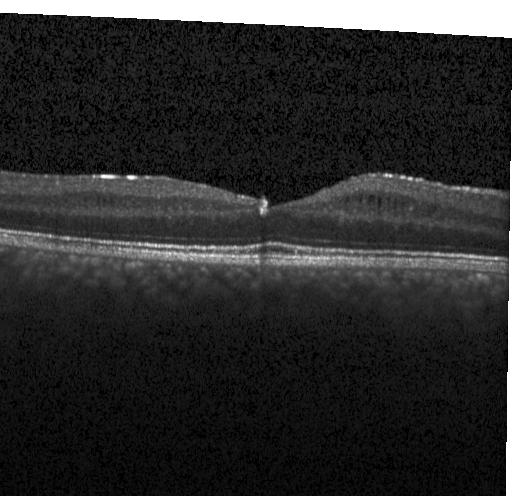
Horizontal scan through the fovea, OCT B-scan, Heidelberg Spectralis OCT system
DME.